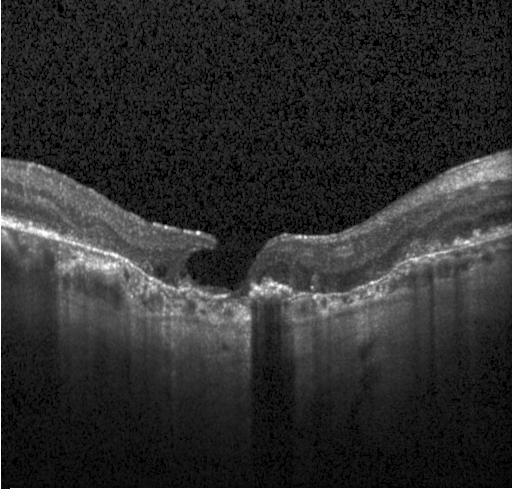

Centered on the fovea, SD-OCT, retinal OCT cross-section, Heidelberg Spectralis OCT system.
Impression: a choroidal neovascular membrane.